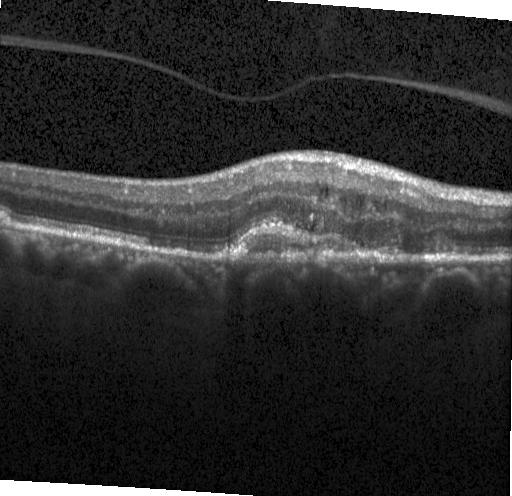
Diagnosis: choroidal neovascularization.